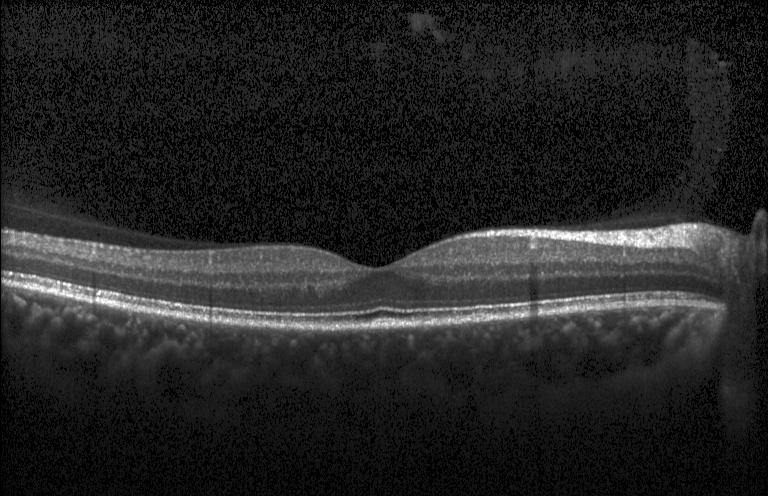

Heidelberg Spectralis OCT system. Optical coherence tomography B-scan. Through the macula
Finding: no choroidal neovascularization, diabetic macular edema, or drusen.